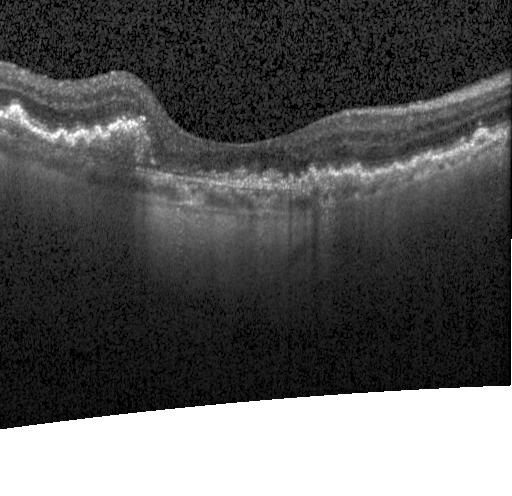
OCT line scan
Choroidal neovascularization (CNV).